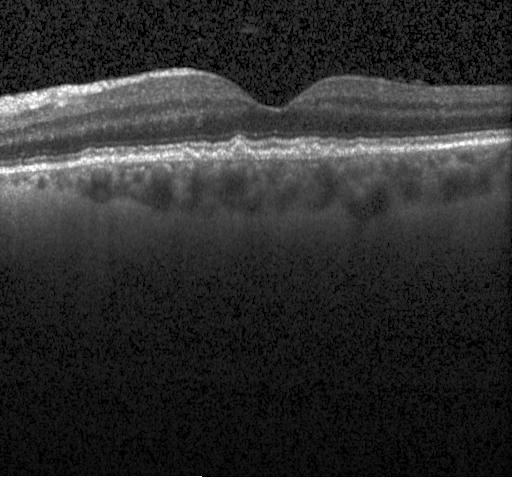 Impression: sub-RPE drusenoid deposits.